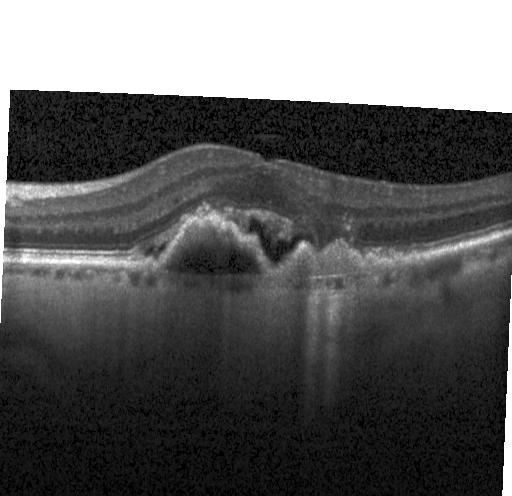
Choroidal neovascularization.